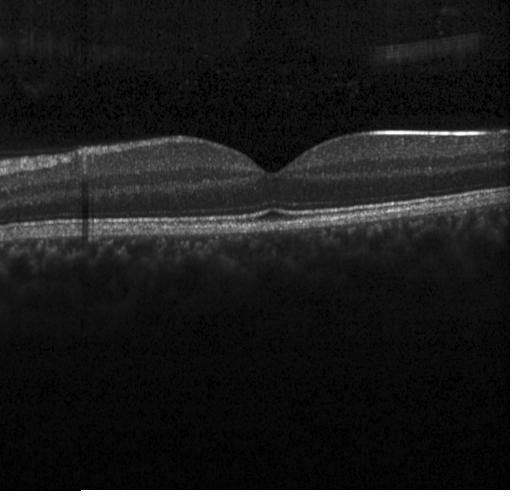

Macular scan, retinal OCT cross-section, spectral-domain OCT.
This B-scan demonstrates no CNV, no DME, and no drusen.